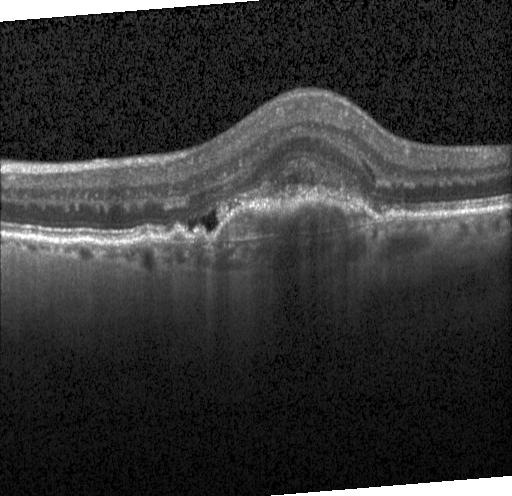 Macular scan, spectral-domain OCT, Heidelberg Spectralis, retinal OCT cross-section. Finding: a choroidal neovascular membrane.